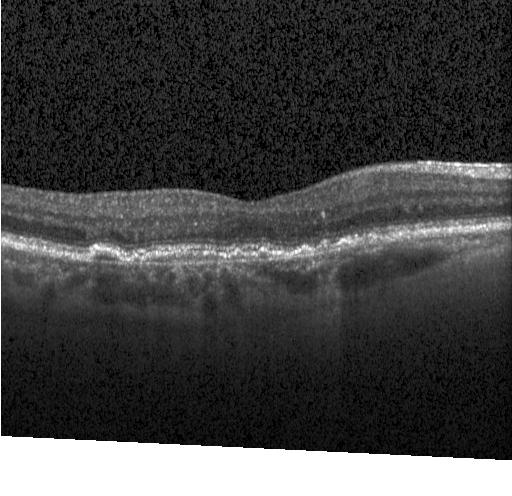

Optical coherence tomography B-scan; Heidelberg Spectralis OCT system — This B-scan demonstrates a choroidal neovascular membrane.